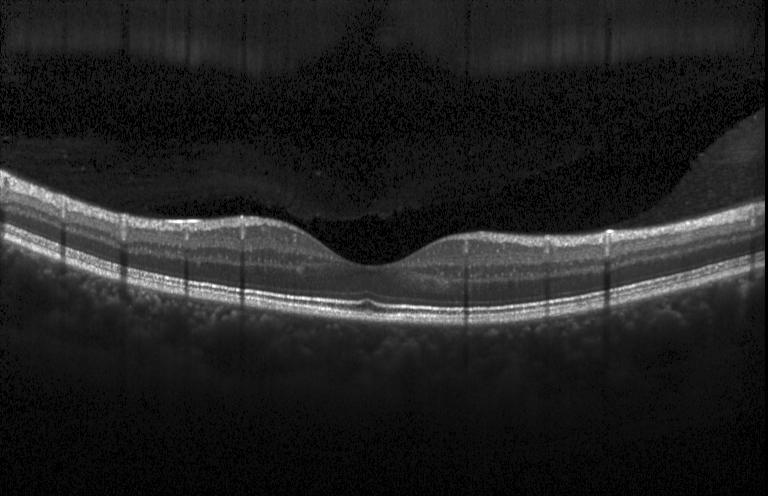

OCT finding: no CNV, DME, or drusen.